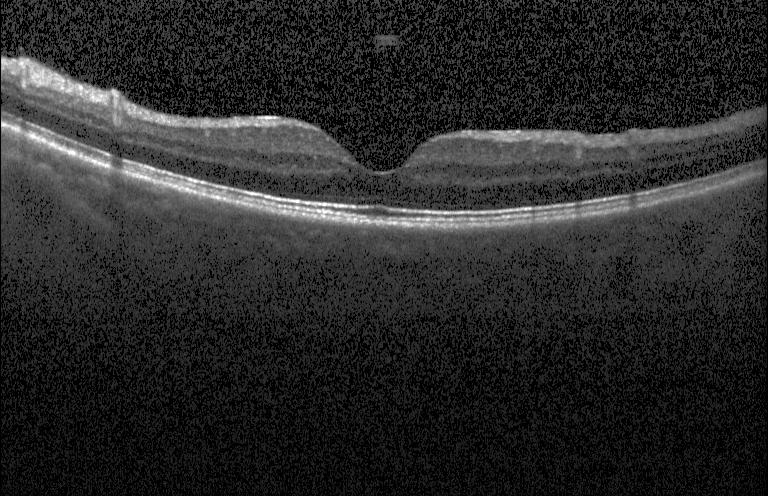
Assessment: no evidence of choroidal neovascularization, diabetic macular edema, or drusen.